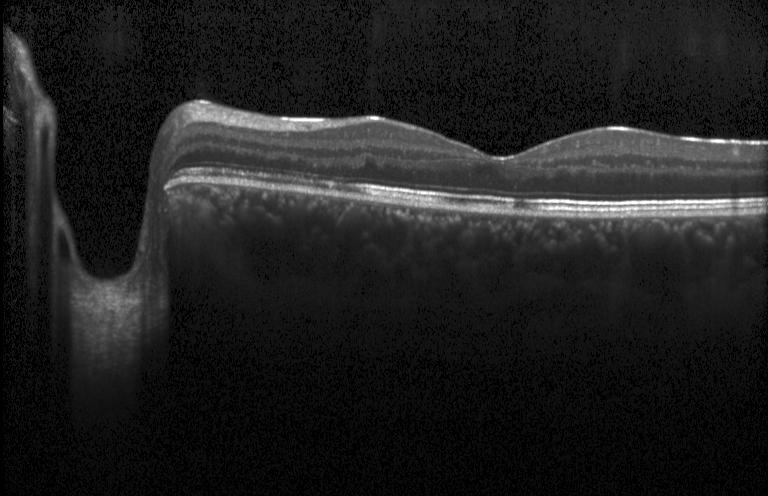
OCT finding: no choroidal neovascularization, no diabetic macular edema, and no drusen.